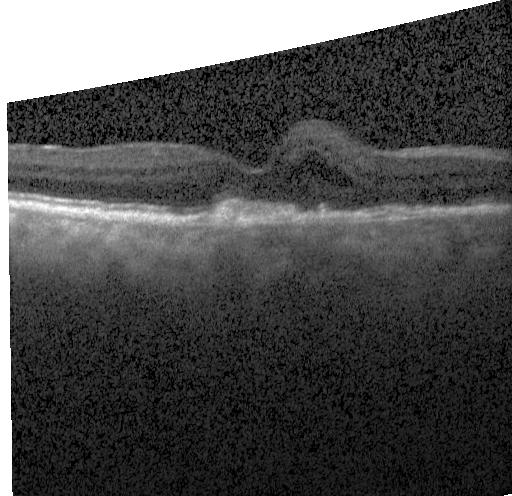

OCT line scan.
CNV.